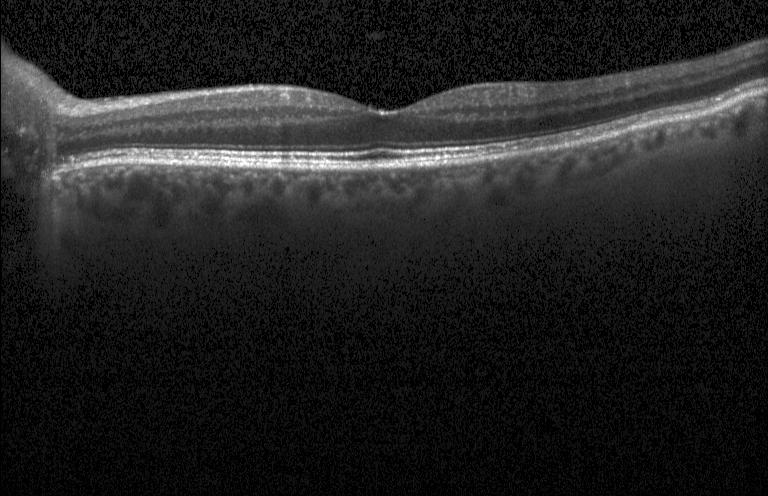
Optical coherence tomography B-scan. Macular scan.
Macular OCT: neither choroidal neovascularization, diabetic macular edema, nor drusen.